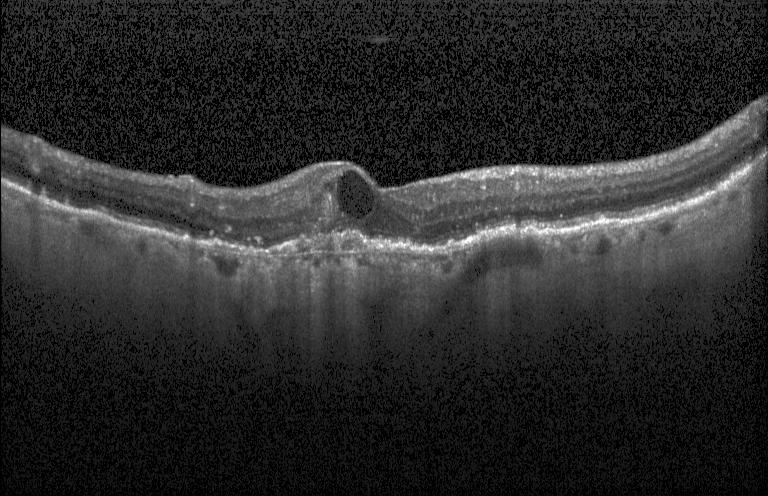
Horizontal scan through the fovea · instrument: Heidelberg Spectralis · OCT line scan — Impression: a choroidal neovascular membrane.